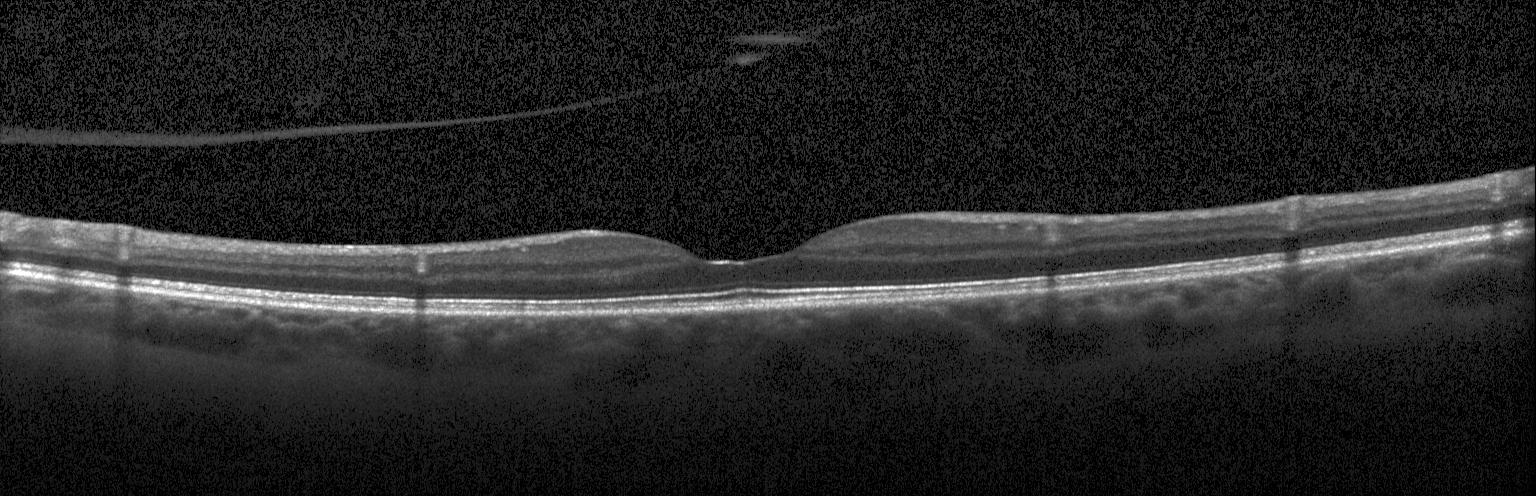

Finding: neither choroidal neovascularization, diabetic macular edema, nor drusen.